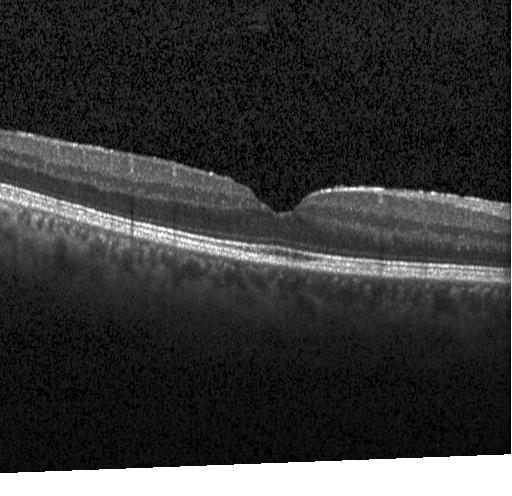
Finding: neither CNV, DME, nor drusen.